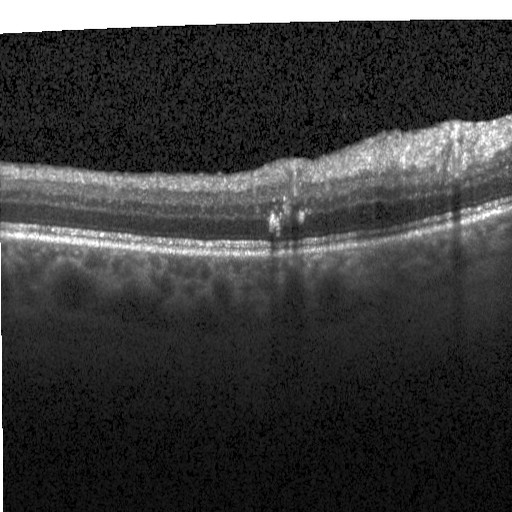
Instrument: Heidelberg Spectralis. Optical coherence tomography scan — Diabetic macular edema.